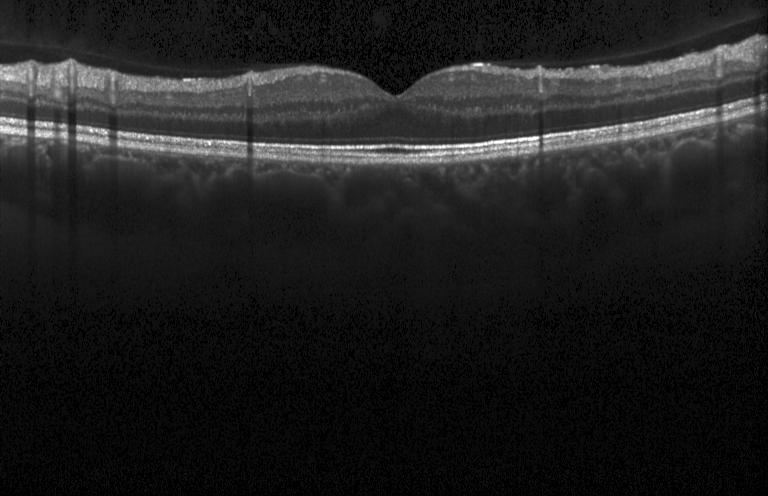
Through the macula, optical coherence tomography scan — OCT finding: no evidence of choroidal neovascularization, diabetic macular edema, or drusen.